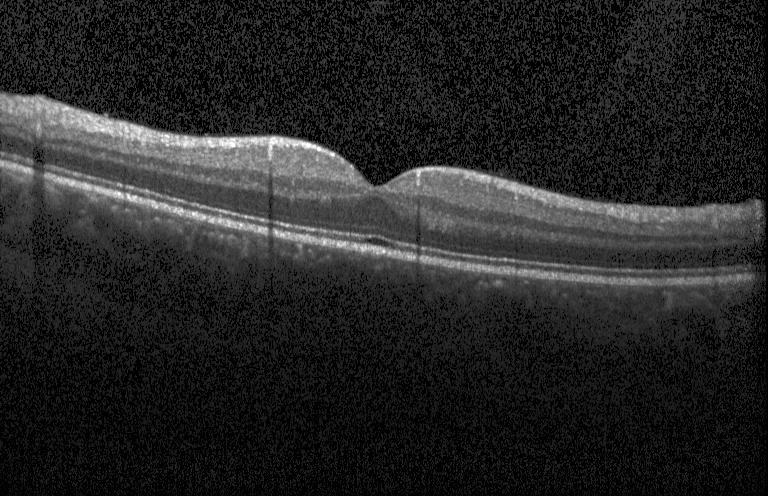
OCT finding: no choroidal neovascularization, no diabetic macular edema, and no drusen.